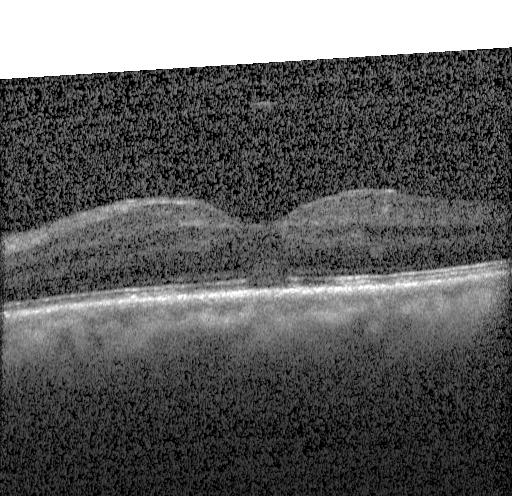

OCT finding: choroidal neovascularization (CNV).